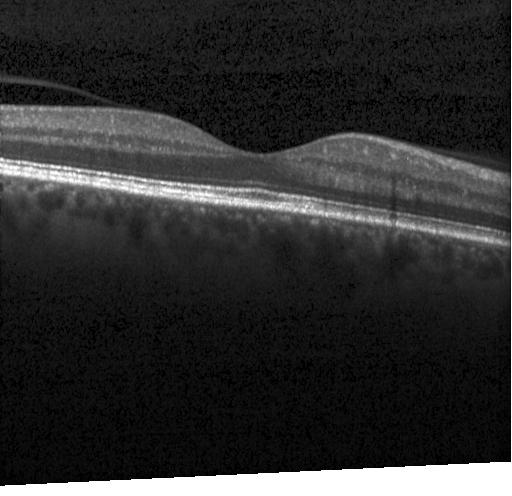 Heidelberg Spectralis OCT system, SD-OCT, horizontal scan through the fovea, retinal OCT cross-section.
This B-scan demonstrates no evidence of choroidal neovascularization, diabetic macular edema, or drusen.